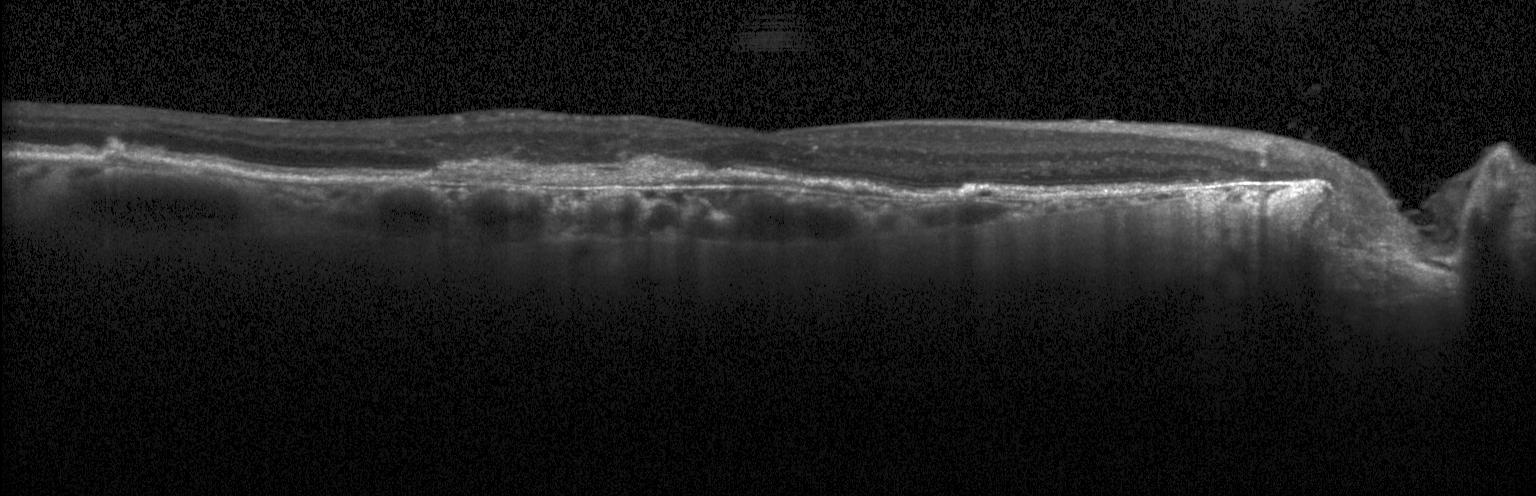

Dx: choroidal neovascularization (CNV).